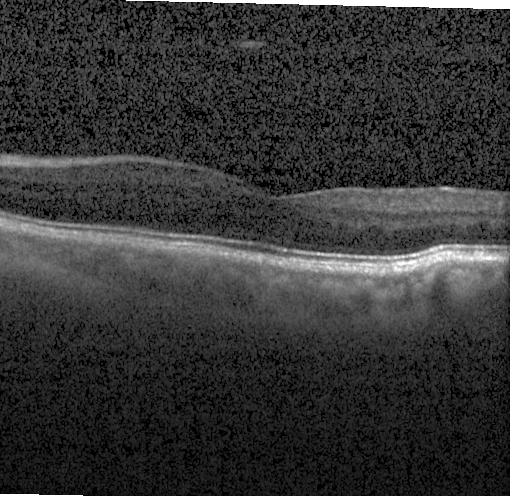
Impression: no CNV, DME, or drusen.